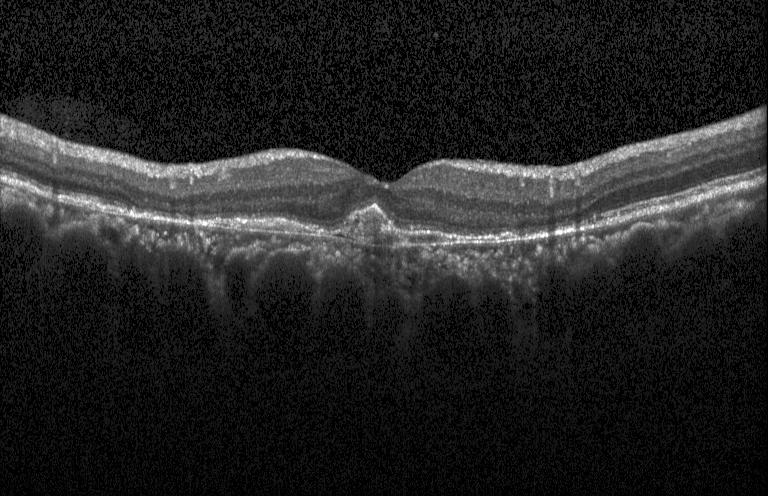

Acquired on a Heidelberg Spectralis; retinal OCT B-scan; spectral-domain OCT
Assessment: CNV.